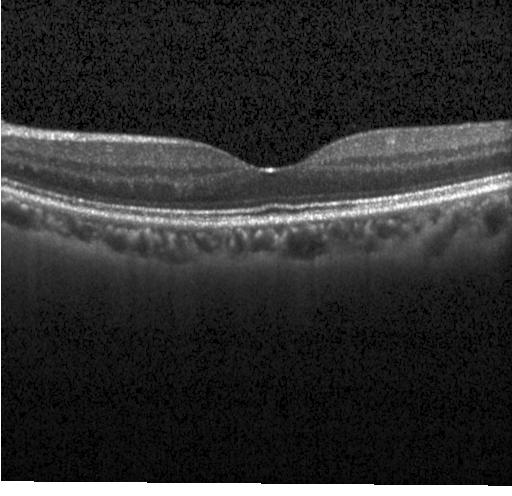
Finding: no choroidal neovascularization, diabetic macular edema, or drusen.